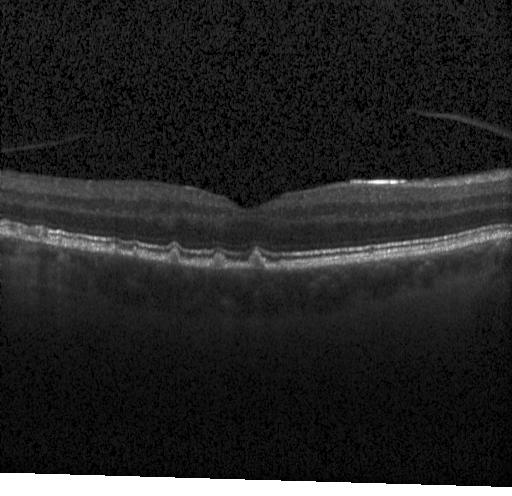

Impression: sub-RPE drusenoid deposits.